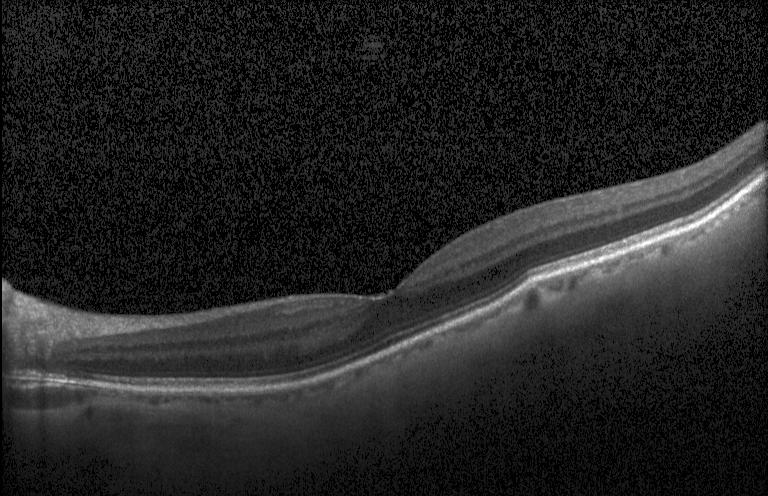

Optical coherence tomography B-scan. The scan shows no evidence of CNV, DME, or drusen.